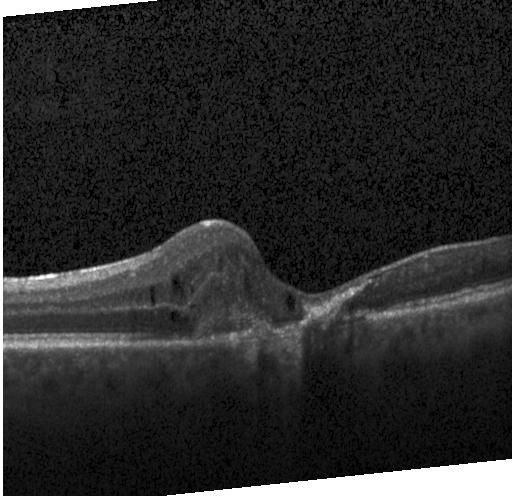

Spectral-domain OCT. Optical coherence tomography B-scan
Finding: a choroidal neovascular membrane.